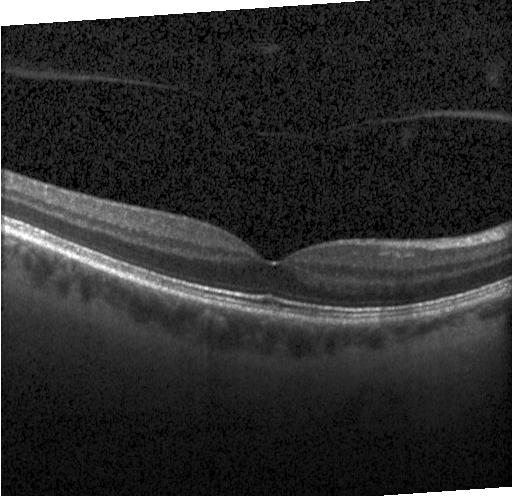
Impression: no choroidal neovascularization, no diabetic macular edema, and no drusen.